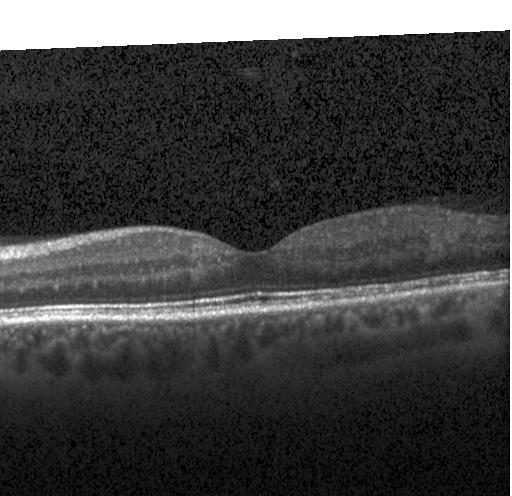
OCT line scan
Impression: no CNV, DME, or drusen.